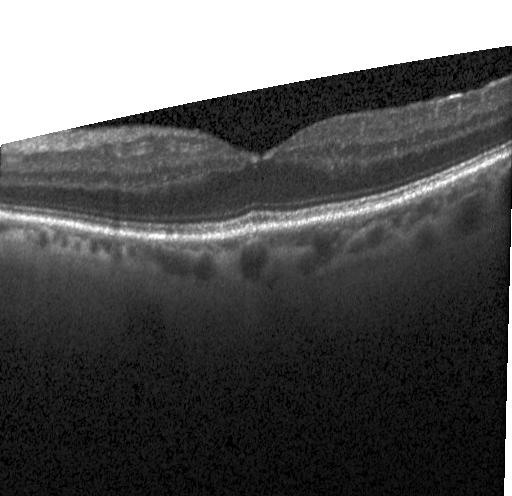
Spectral-domain optical coherence tomography; Heidelberg Spectralis OCT system; OCT B-scan; macular scan.
Assessment: no evidence of choroidal neovascularization, diabetic macular edema, or drusen.